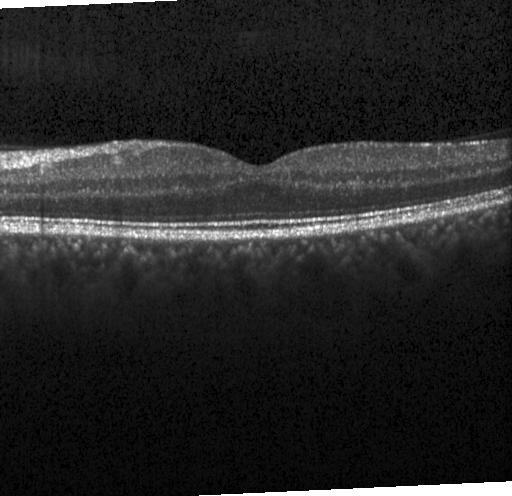

Impression: no evidence of CNV, DME, or drusen.